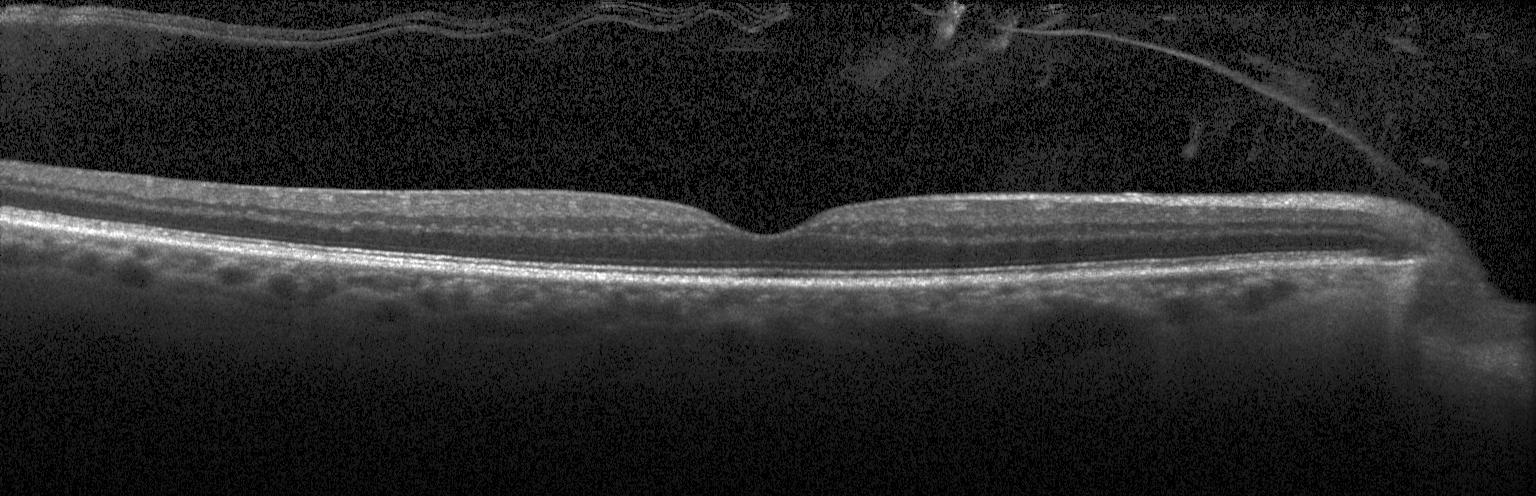

Optical coherence tomography B-scan, Heidelberg Spectralis OCT system, SD-OCT — Macular OCT: no evidence of choroidal neovascularization, diabetic macular edema, or drusen.